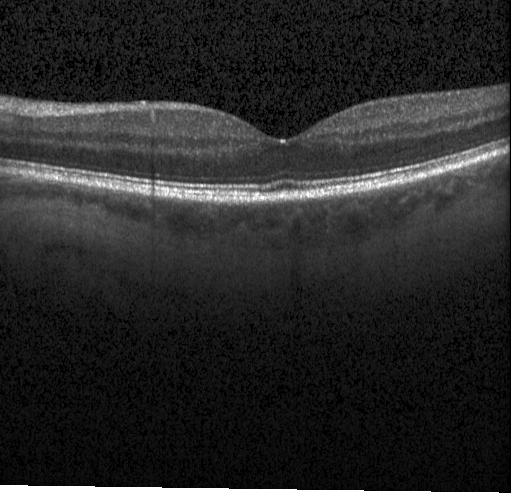
OCT finding: neither choroidal neovascularization, diabetic macular edema, nor drusen.